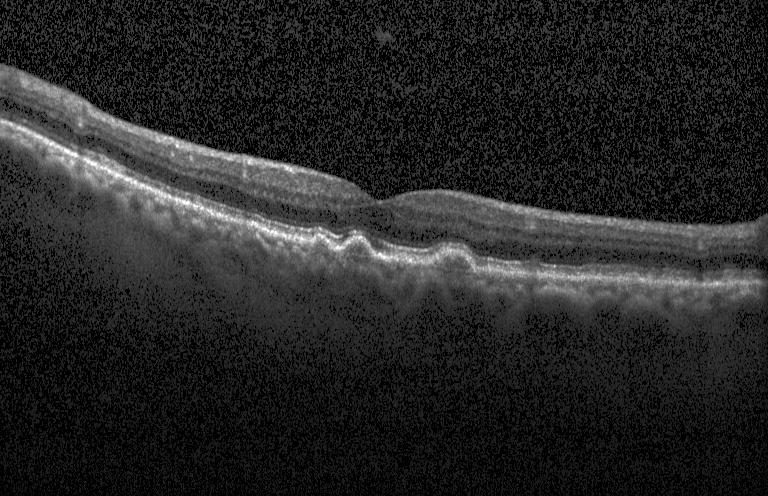

This B-scan demonstrates drusen.